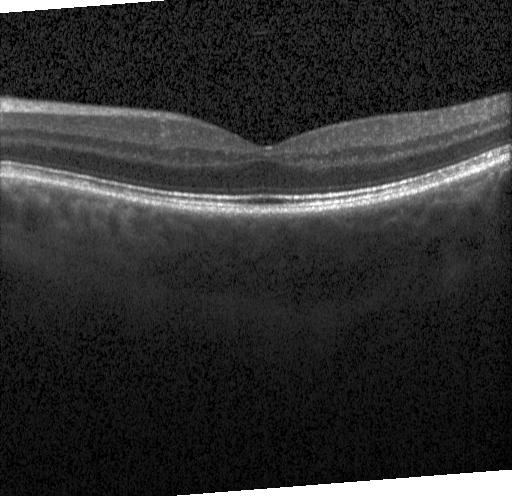 OCT line scan. Impression: neither CNV, DME, nor drusen.